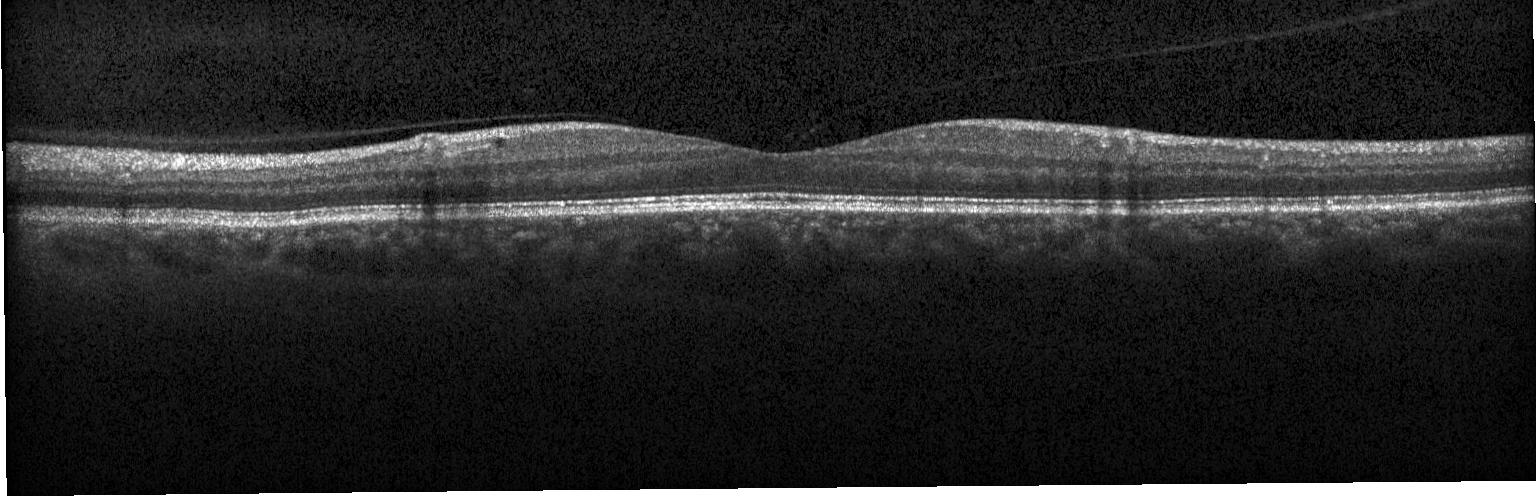
No evidence of choroidal neovascularization, diabetic macular edema, or drusen.